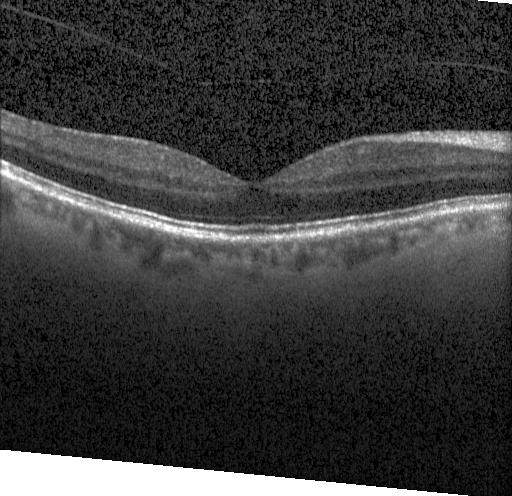

Macular OCT: neither choroidal neovascularization, diabetic macular edema, nor drusen.